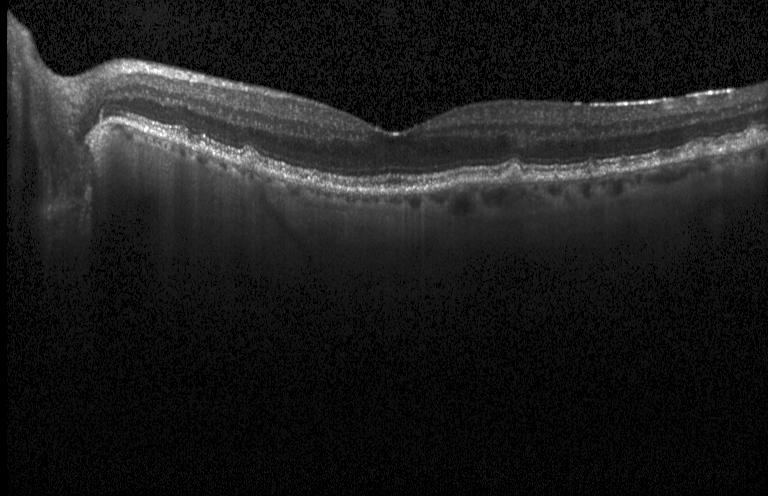
Centered on the fovea, optical coherence tomography scan, spectral-domain optical coherence tomography, Heidelberg Spectralis. Macular OCT: multiple drusen.